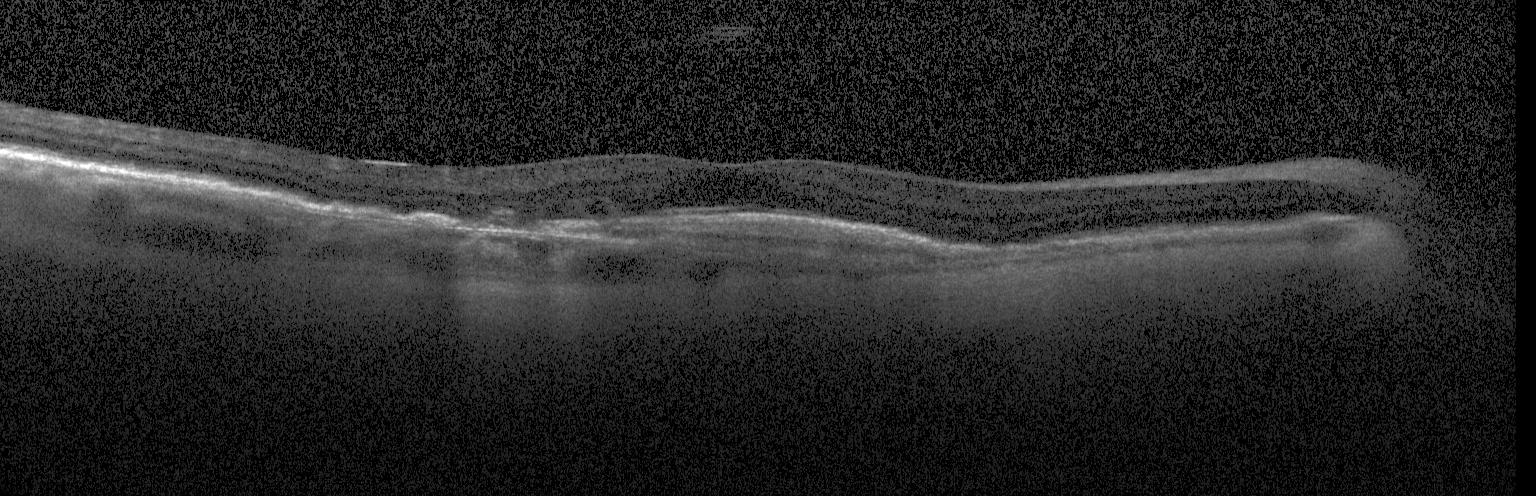

Macular OCT demonstrating choroidal neovascularization (CNV).